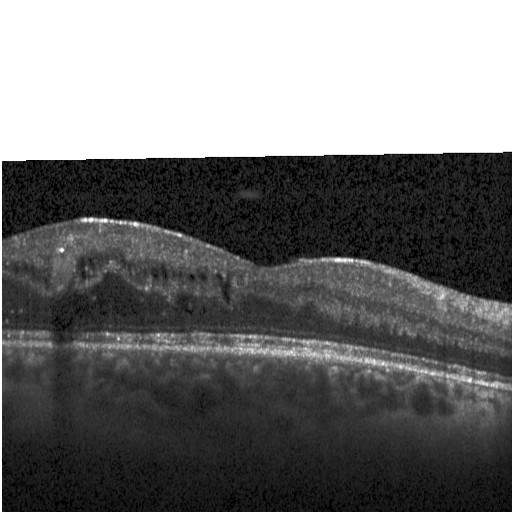 OCT B-scan · SD-OCT · horizontal scan through the fovea.
Diabetic macular edema.